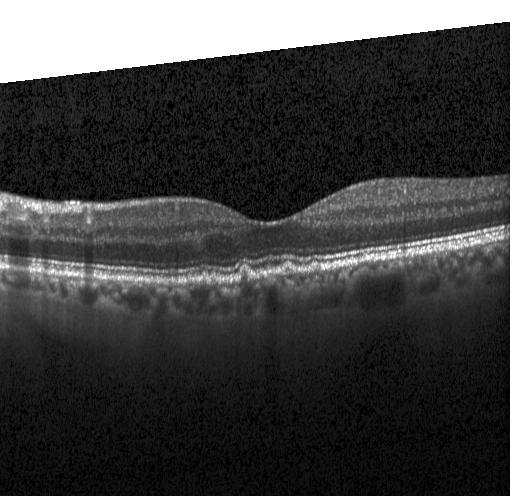 Through the macula · OCT B-scan · spectral-domain optical coherence tomography · acquired on a Heidelberg Spectralis.
Assessment: sub-RPE drusenoid deposits.